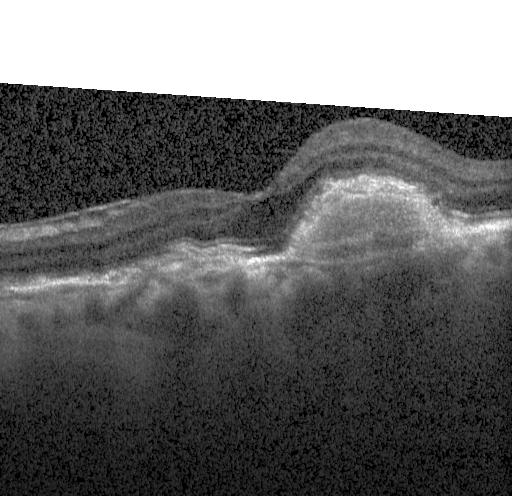 The scan shows a choroidal neovascular membrane.